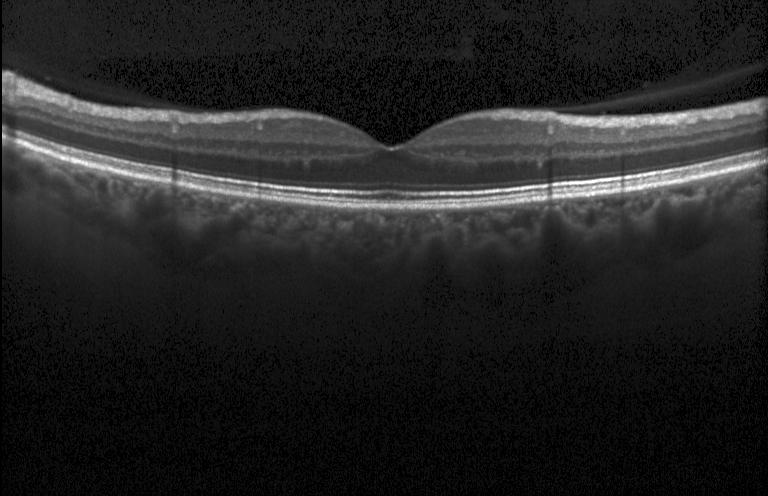
Retinal OCT cross-section
Finding: no CNV, DME, or drusen.